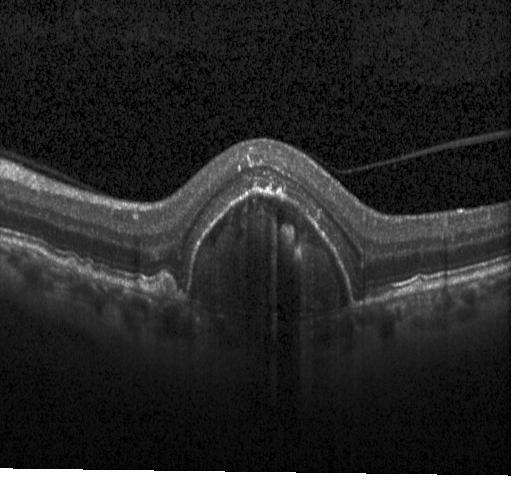
Optical coherence tomography scan, Heidelberg Spectralis OCT system. Diagnosis: a choroidal neovascular membrane.